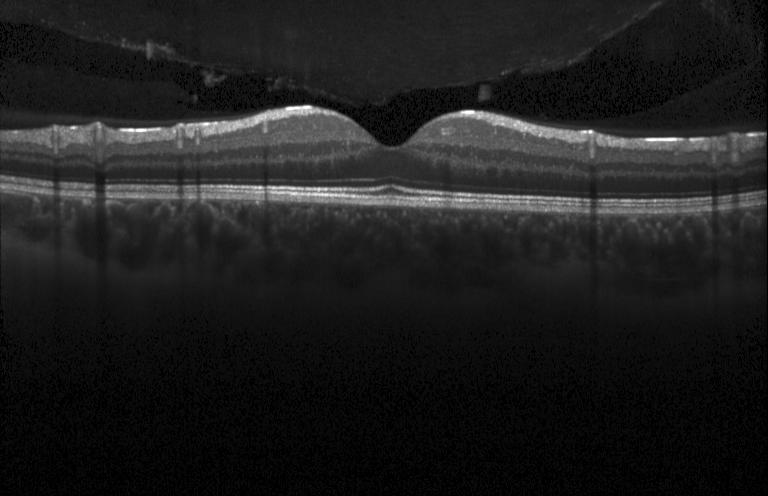 Retinal OCT B-scan.
Impression: no CNV, no DME, and no drusen.